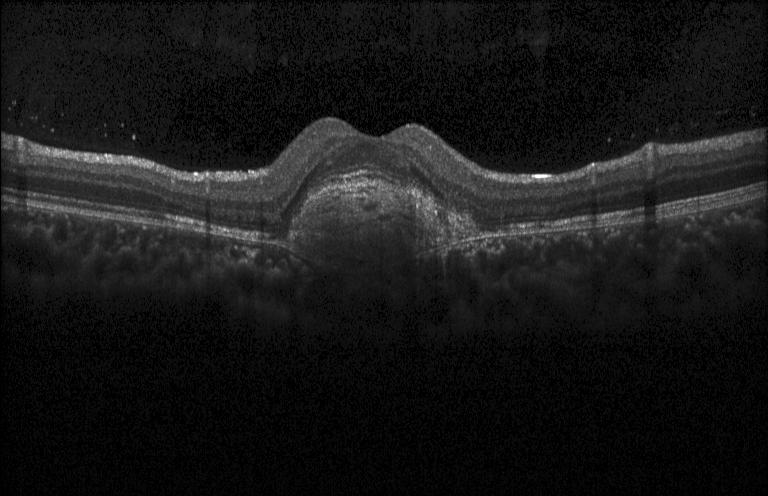 Finding: a choroidal neovascular membrane.